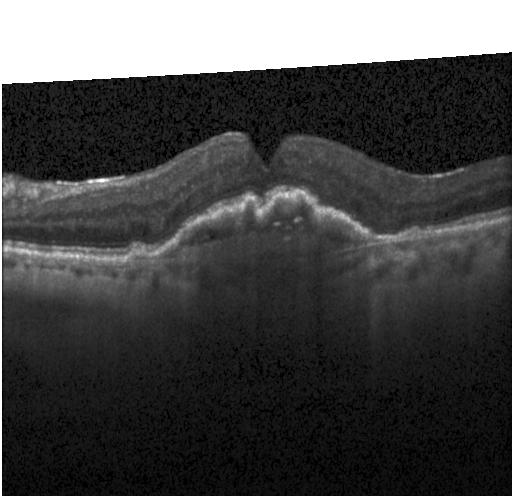
OCT finding: a choroidal neovascular membrane.